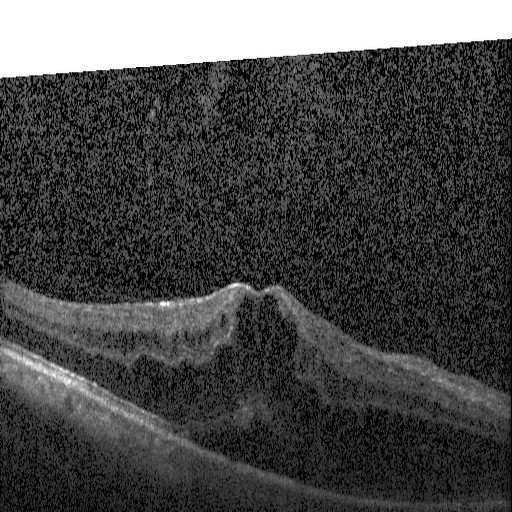 Retinal OCT cross-section showing diabetic macular edema (DME).